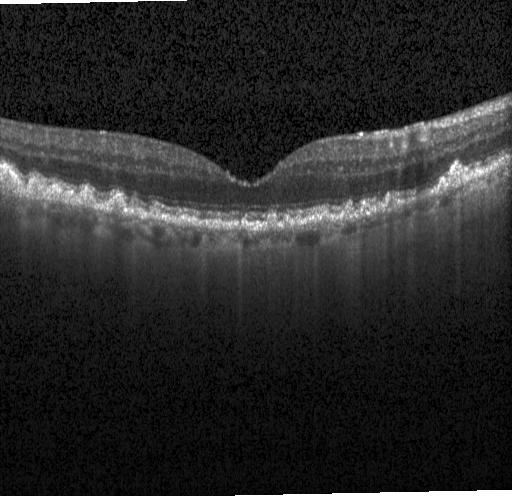 Heidelberg Spectralis OCT system, OCT B-scan. Finding: sub-RPE drusenoid deposits.